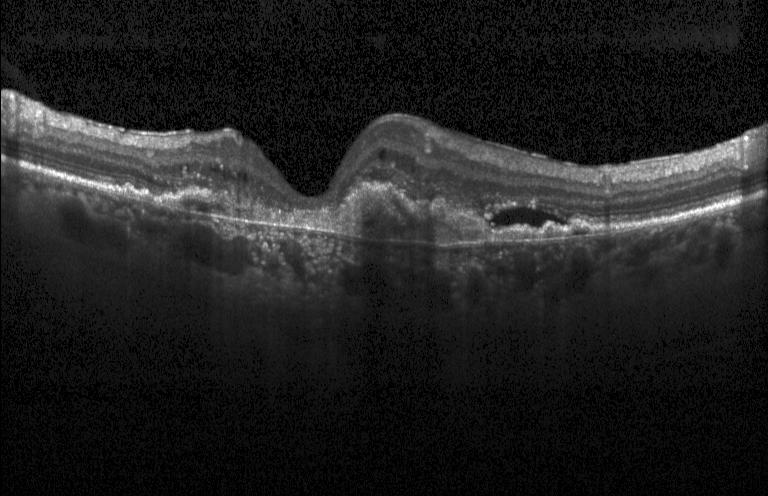
Retinal OCT B-scan, SD-OCT, instrument: Heidelberg Spectralis.
Dx: a choroidal neovascular membrane.